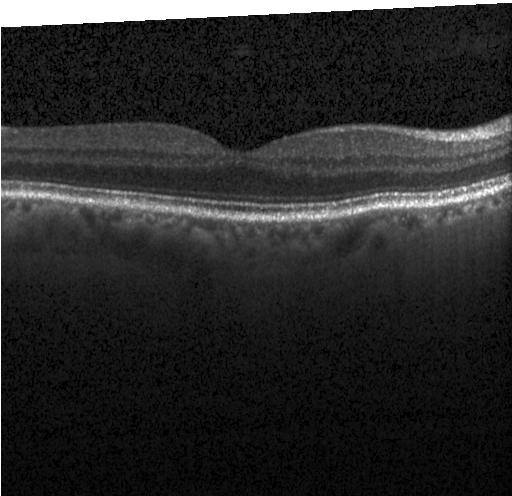 Dx: no CNV, no DME, and no drusen.